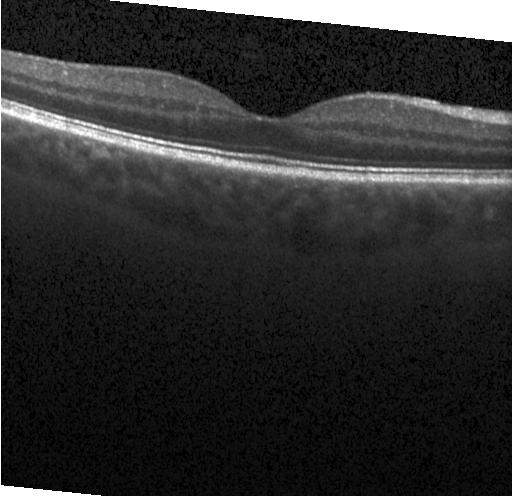

OCT B-scan
Finding: neither choroidal neovascularization, diabetic macular edema, nor drusen.